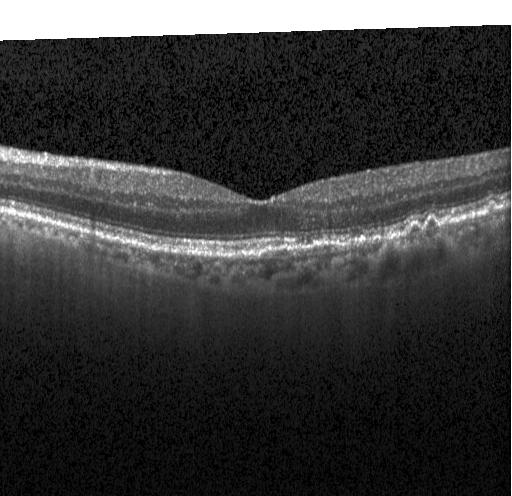
Finding: multiple drusen.